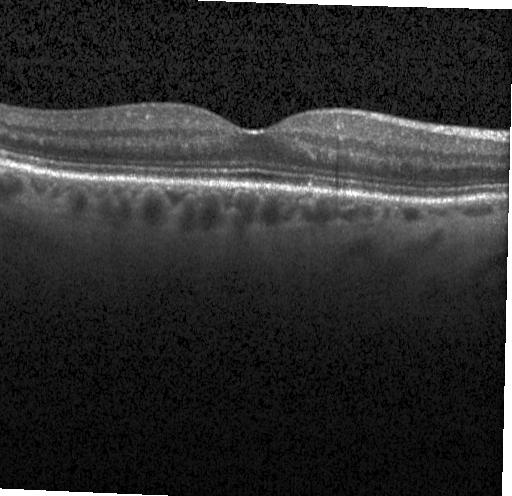

Spectral-domain OCT B-scan: no choroidal neovascularization, no diabetic macular edema, and no drusen.